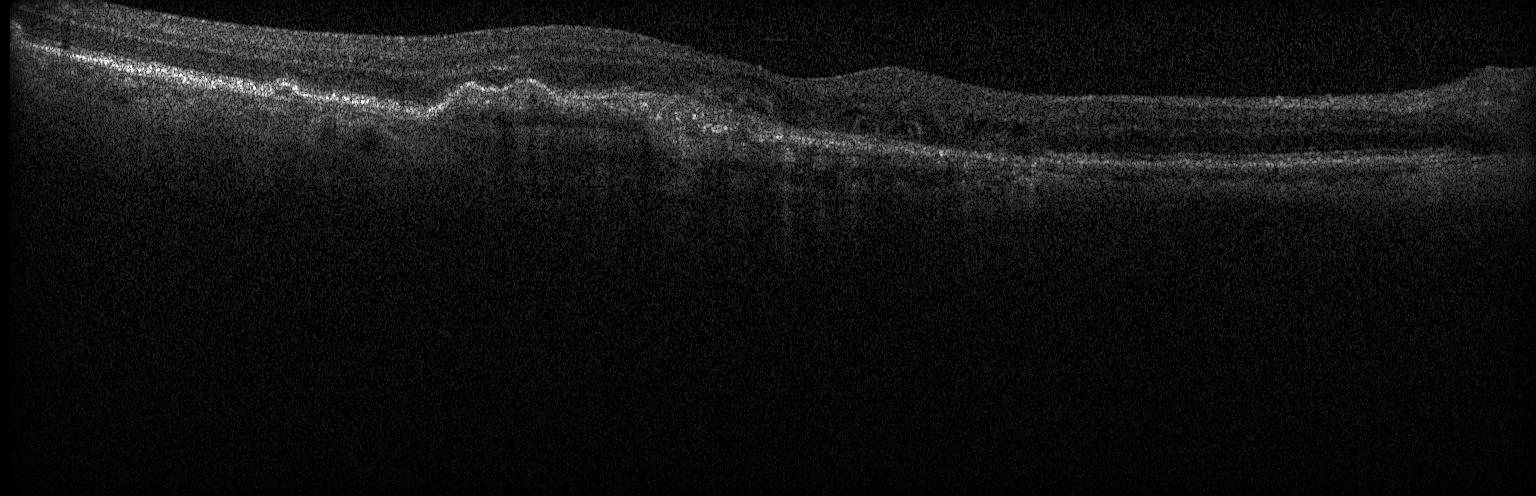 Spectral-domain OCT B-scan: a choroidal neovascular membrane.